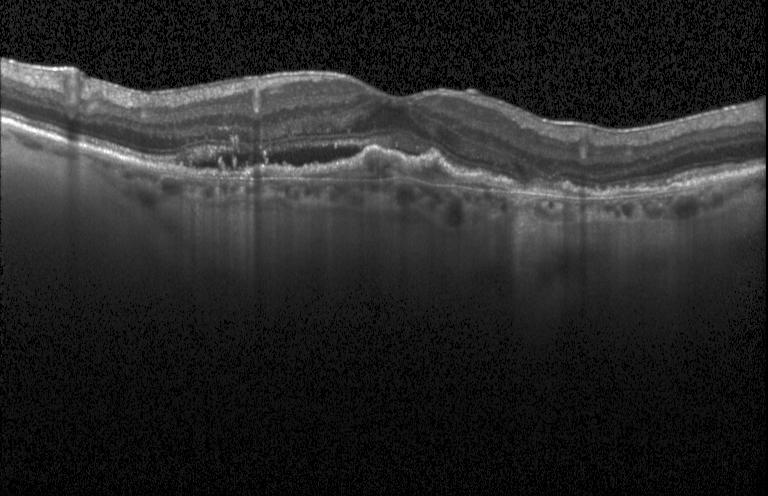
Finding: CNV.